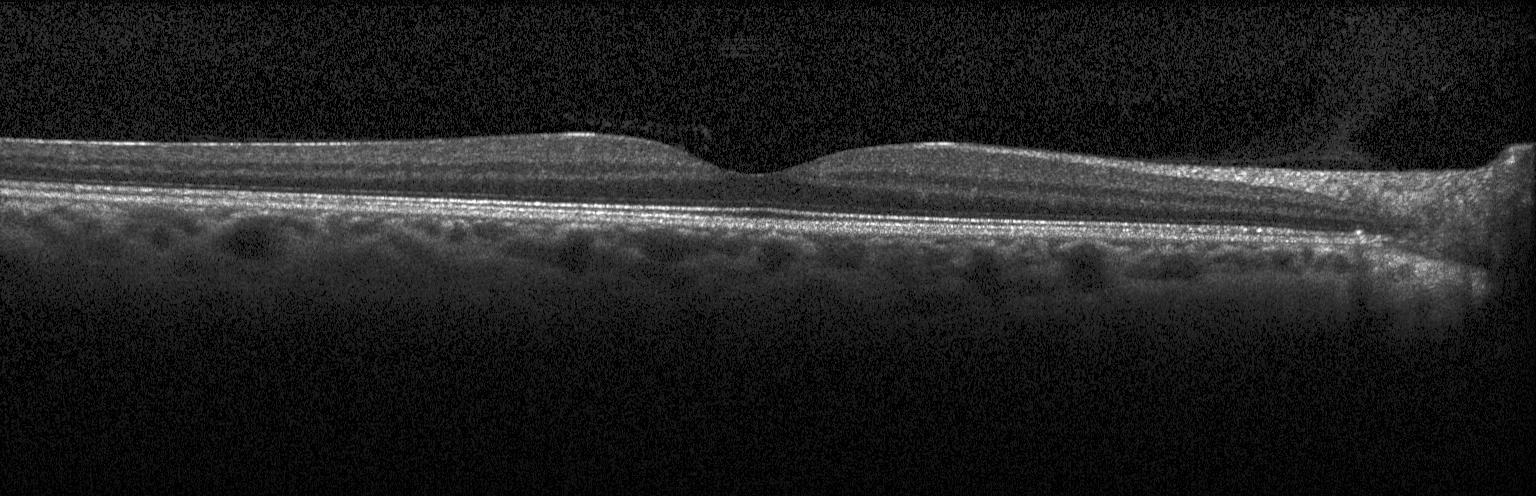 Optical coherence tomography B-scan, Heidelberg Spectralis, SD-OCT. The scan shows no choroidal neovascularization, no diabetic macular edema, and no drusen.